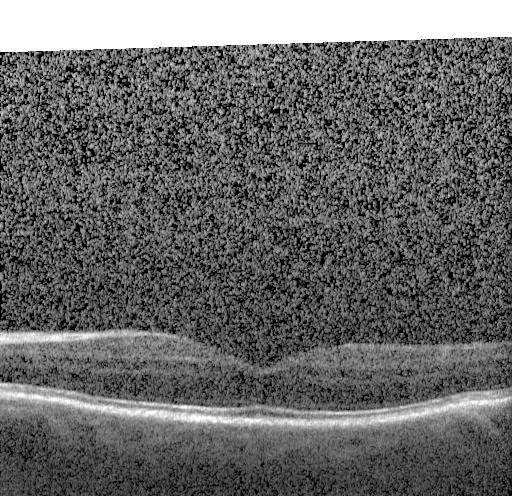 OCT scan showing no evidence of choroidal neovascularization, diabetic macular edema, or drusen.